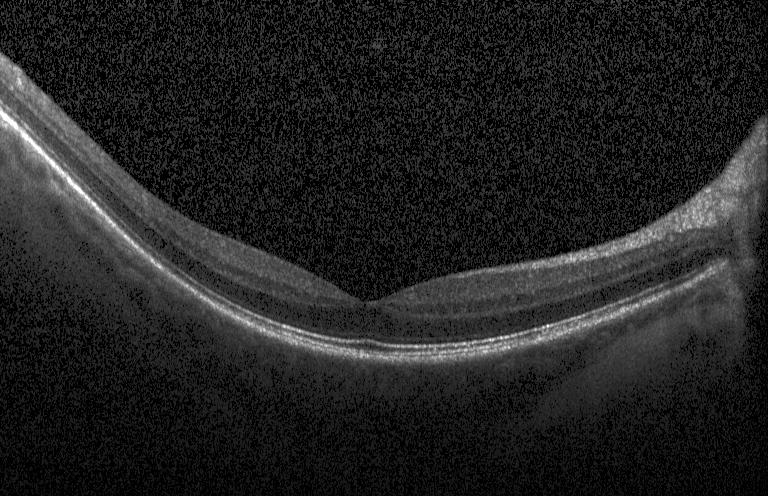
This B-scan demonstrates no evidence of choroidal neovascularization, diabetic macular edema, or drusen.